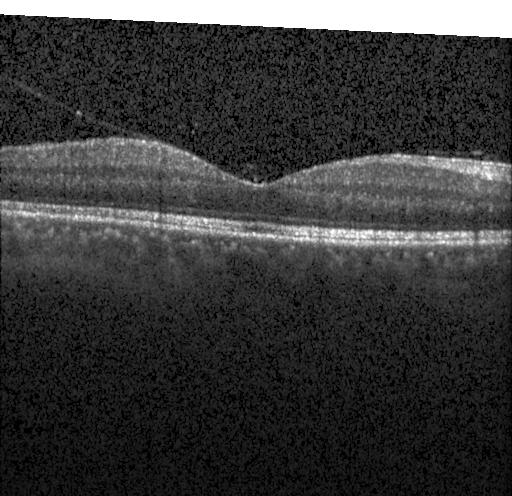 This B-scan demonstrates no evidence of choroidal neovascularization, diabetic macular edema, or drusen.